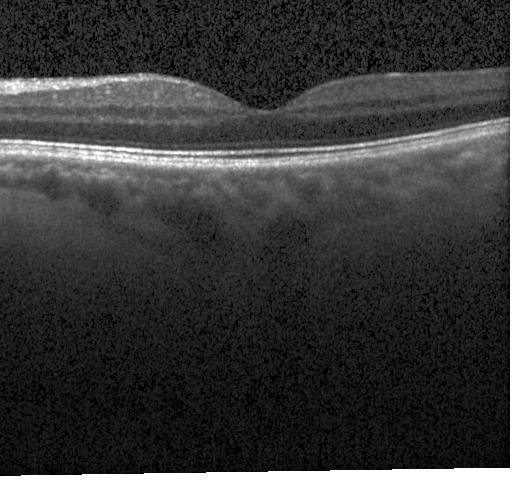 Spectral-domain optical coherence tomography. Horizontal scan through the fovea. Heidelberg Spectralis. Optical coherence tomography scan.
Dx: no evidence of choroidal neovascularization, diabetic macular edema, or drusen.